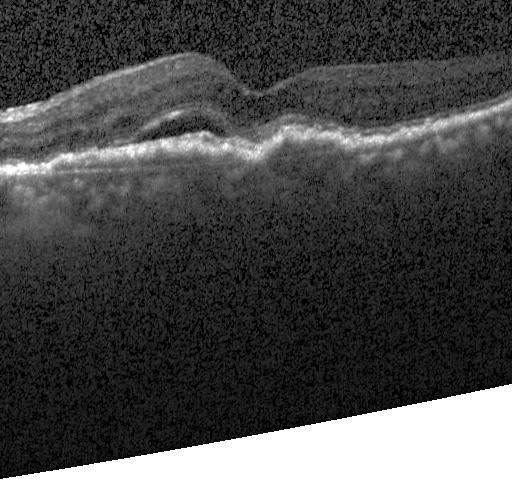
Optical coherence tomography B-scan. Assessment: a choroidal neovascular membrane.